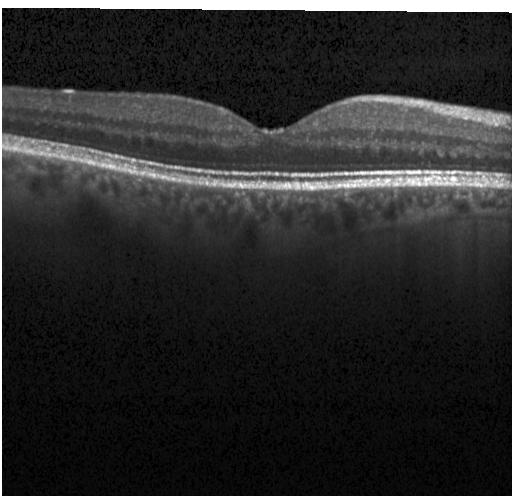

OCT line scan. Spectral-domain optical coherence tomography — Macular OCT: no choroidal neovascularization, diabetic macular edema, or drusen.